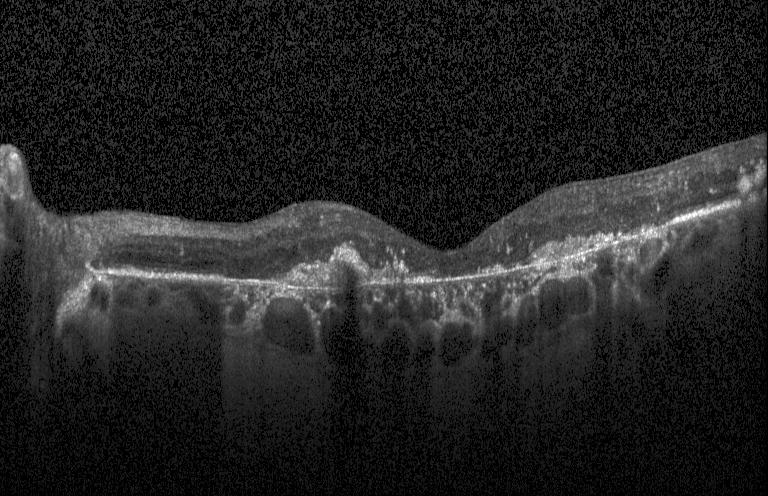
Optical coherence tomography scan; through the macula
Finding: CNV.